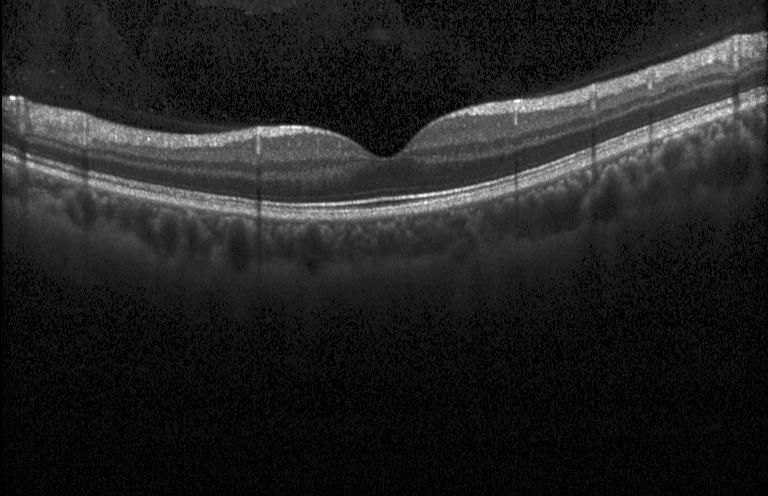
Macular OCT: no evidence of CNV, DME, or drusen.